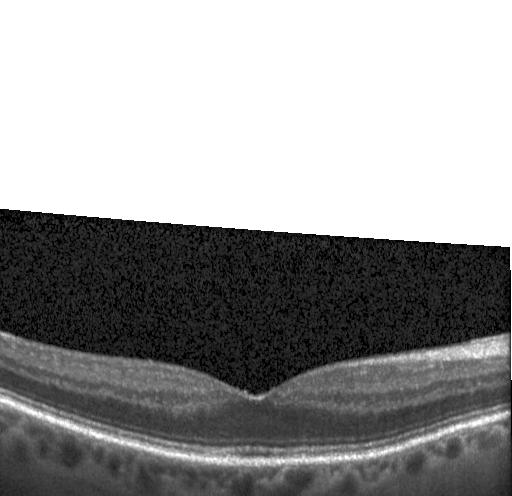 Macular OCT: no CNV, DME, or drusen.